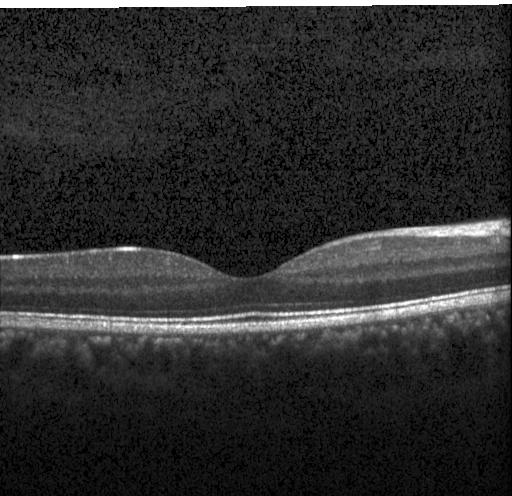

Heidelberg Spectralis OCT system · OCT B-scan — OCT finding: no choroidal neovascularization, no diabetic macular edema, and no drusen.